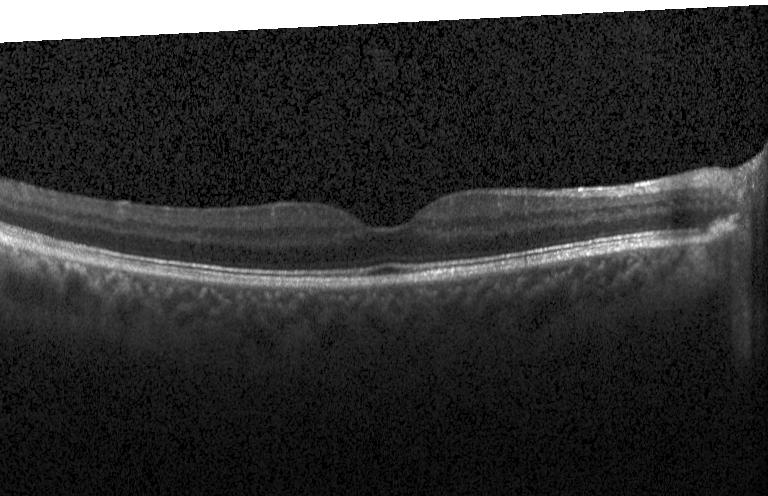

Finding: neither choroidal neovascularization, diabetic macular edema, nor drusen.